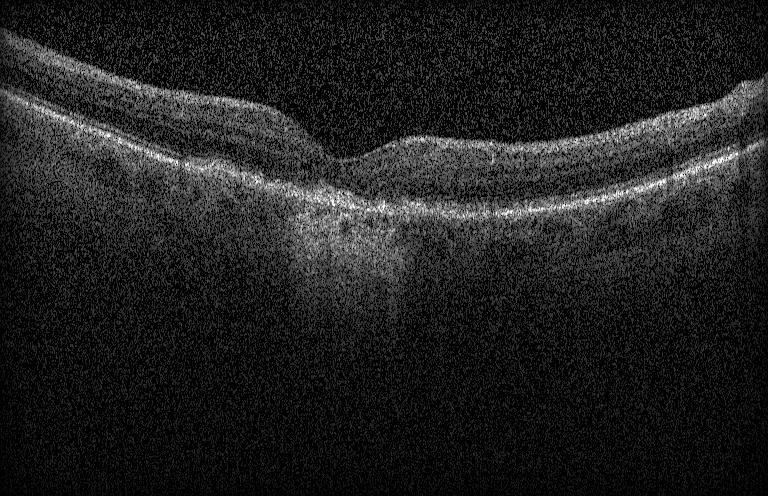
Impression: choroidal neovascularization.